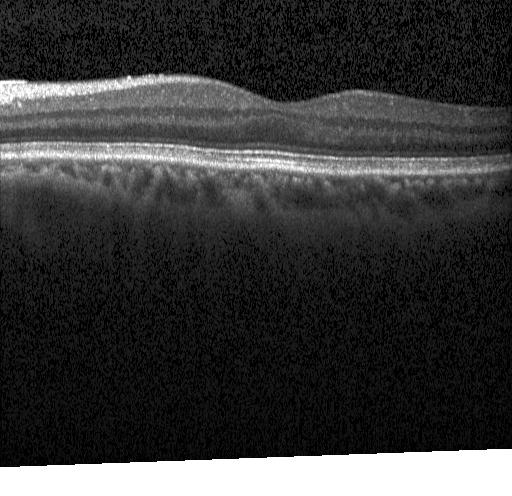

Macular OCT demonstrating neither CNV, DME, nor drusen.